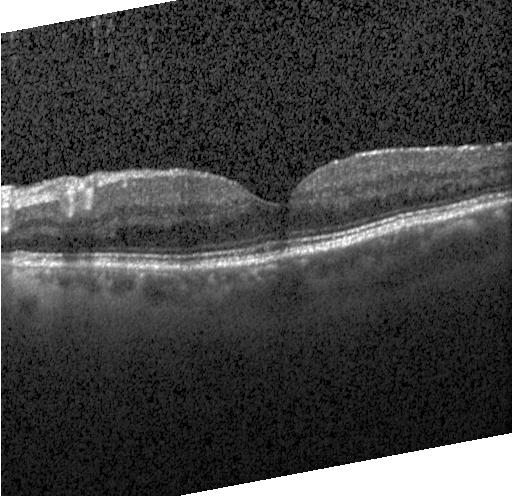
Through the macula. OCT line scan. SD-OCT. Heidelberg Spectralis OCT system. No evidence of choroidal neovascularization, diabetic macular edema, or drusen.